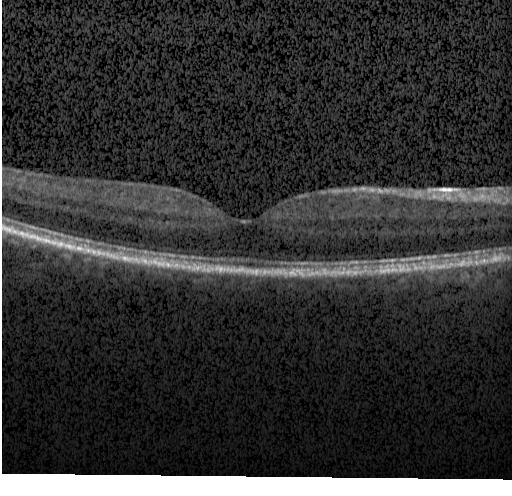 Fovea-centered. OCT B-scan. Macular OCT: no choroidal neovascularization, no diabetic macular edema, and no drusen.